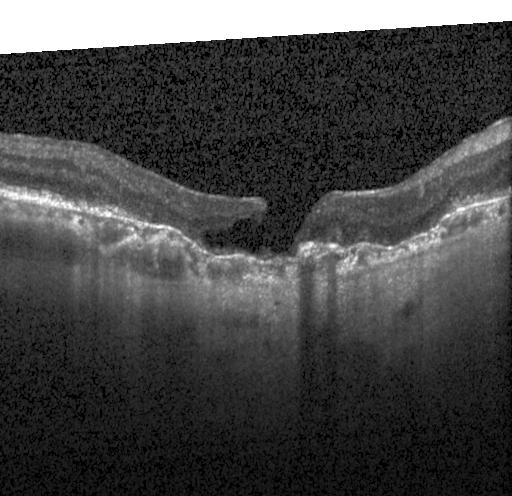
Optical coherence tomography B-scan. Instrument: Heidelberg Spectralis. Macular scan. Spectral-domain OCT. Diagnosis: a choroidal neovascular membrane.